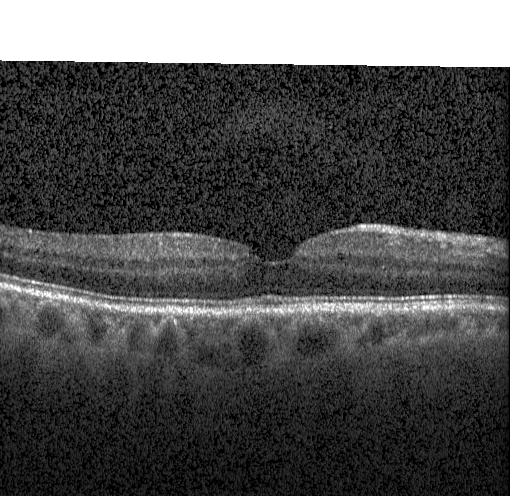 Instrument: Heidelberg Spectralis, OCT line scan, spectral-domain optical coherence tomography — The scan shows no choroidal neovascularization, no diabetic macular edema, and no drusen.